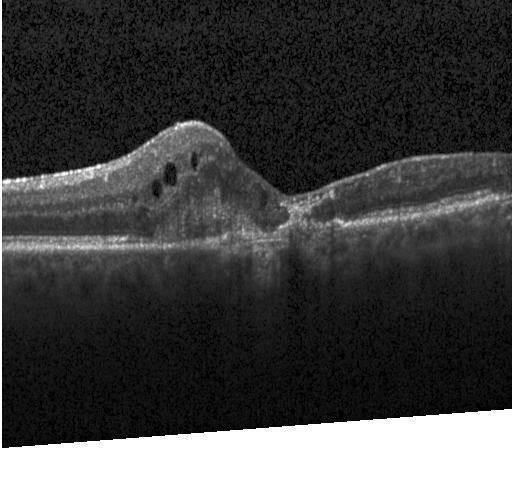 OCT B-scan
Assessment: CNV.